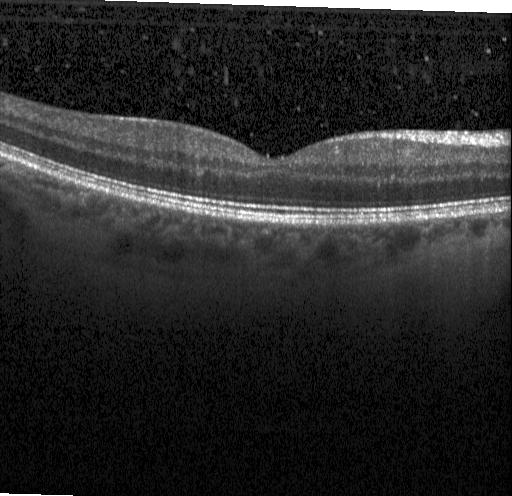 OCT line scan · Heidelberg Spectralis — The scan shows neither choroidal neovascularization, diabetic macular edema, nor drusen.